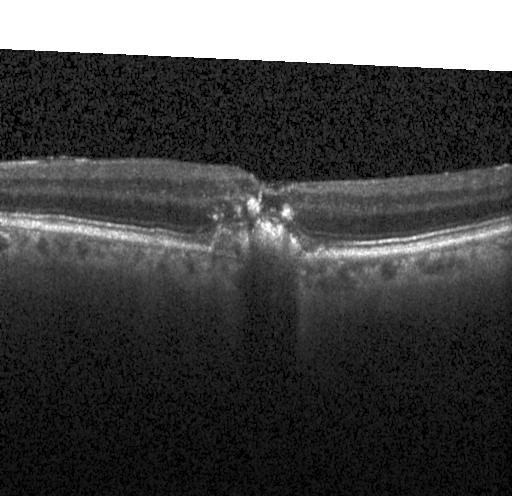 Finding: choroidal neovascularization (CNV).